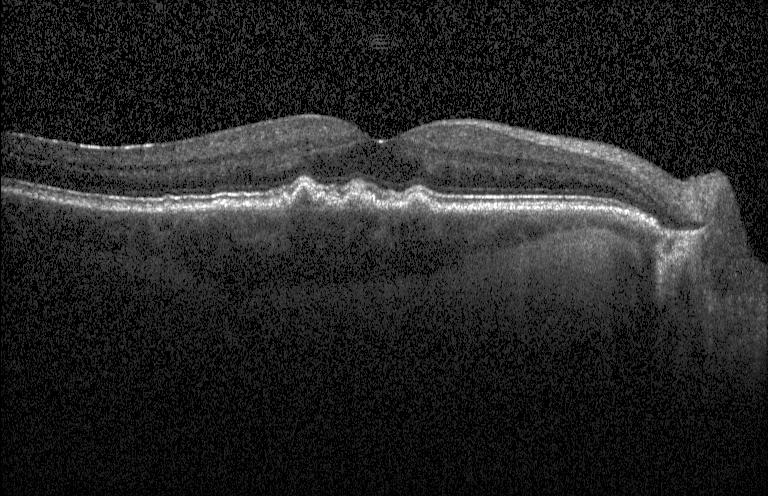

Retinal OCT cross-section showing drusen.